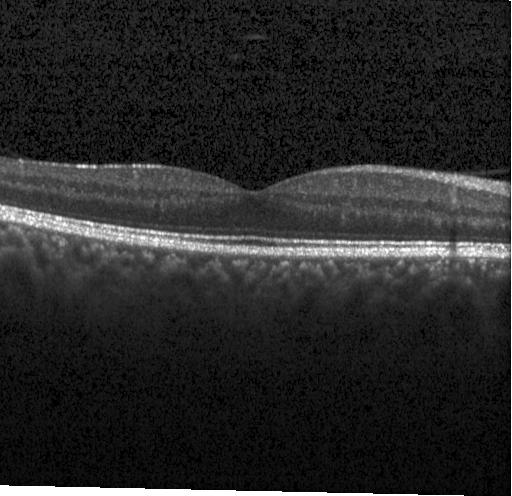

Retinal OCT cross-section; spectral-domain OCT; through the macula; Heidelberg Spectralis OCT system
The scan shows no evidence of choroidal neovascularization, diabetic macular edema, or drusen.